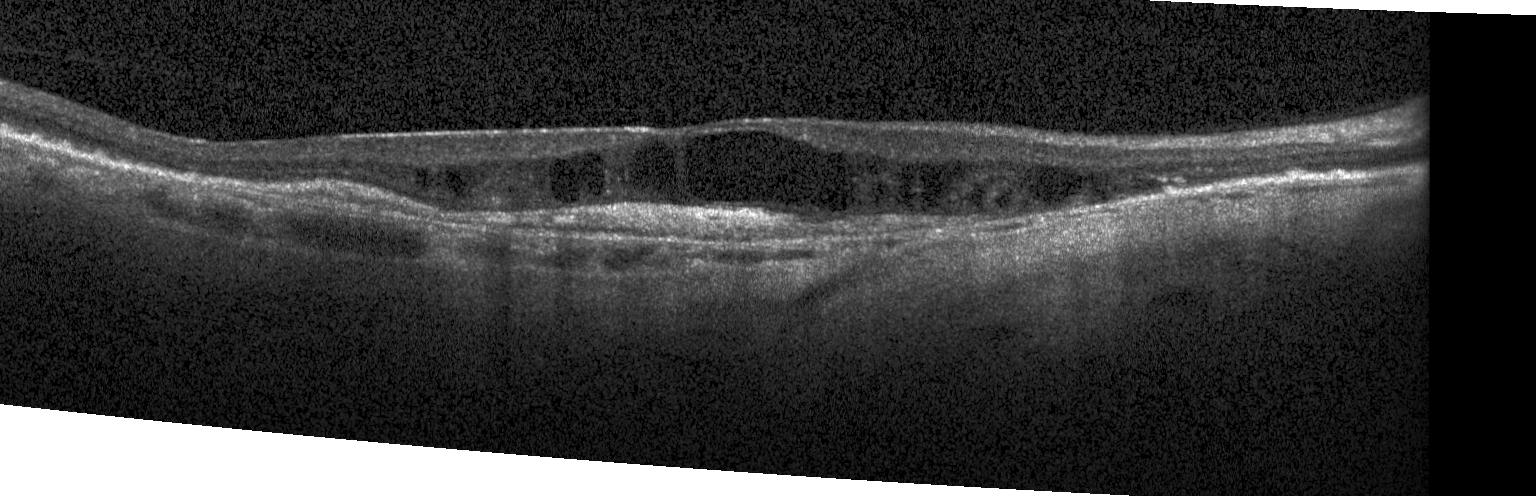 Retinal OCT cross-section; SD-OCT.
Impression: CNV.